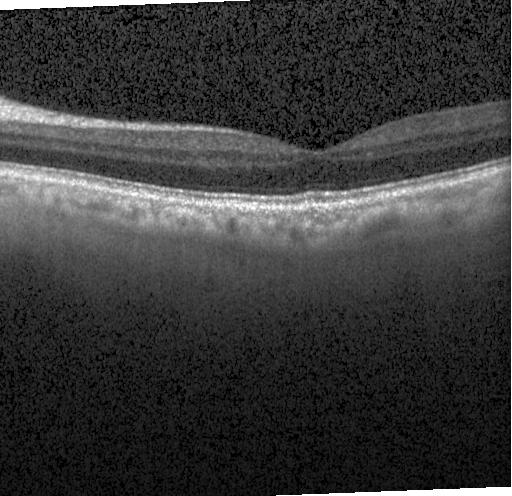 Retinal OCT B-scan · instrument: Heidelberg Spectralis · macular scan · spectral-domain OCT.
Macular OCT: no CNV, no DME, and no drusen.